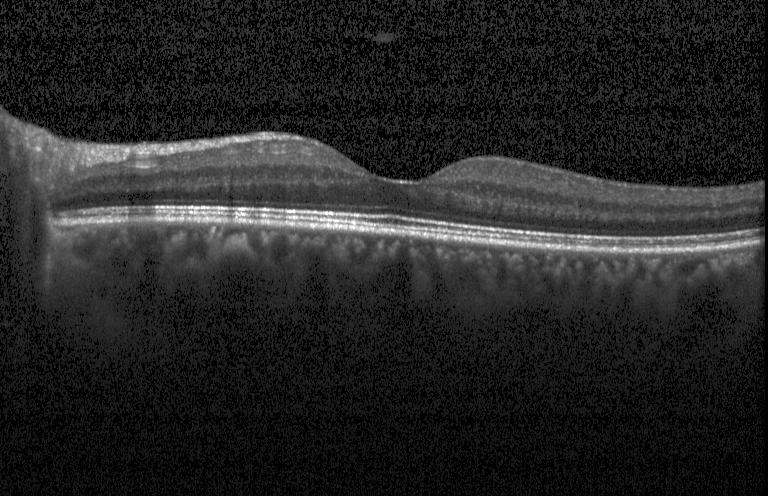
Horizontal scan through the fovea · spectral-domain OCT · retinal OCT B-scan.
OCT finding: no CNV, DME, or drusen.